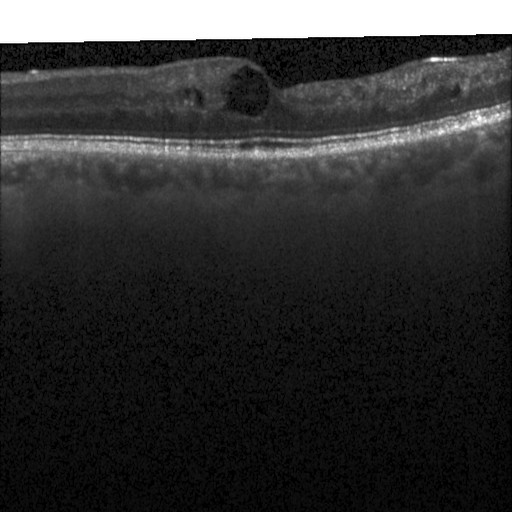

OCT line scan
Finding: diabetic macular edema (DME).